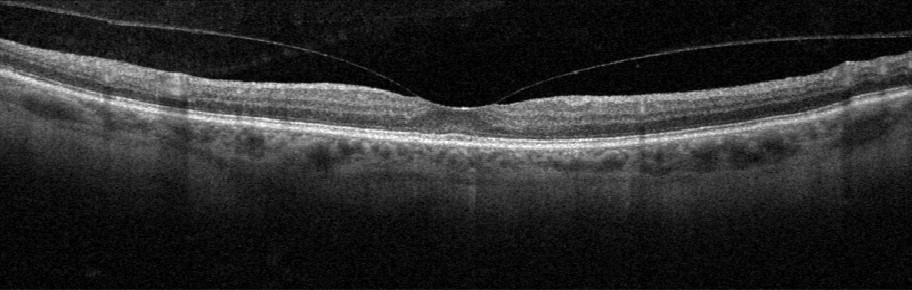 Retinal OCT B-scan — Finding: VID.